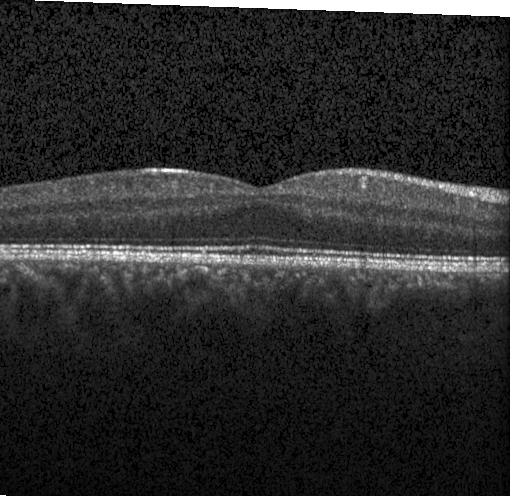
Optical coherence tomography B-scan, spectral-domain OCT
Impression: no choroidal neovascularization, diabetic macular edema, or drusen.